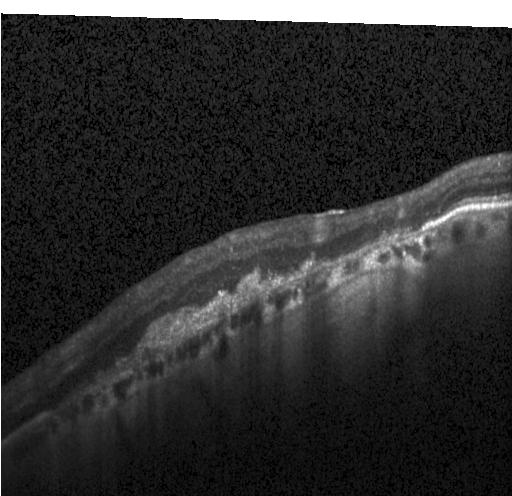 Retinal OCT cross-section — The scan shows a choroidal neovascular membrane.